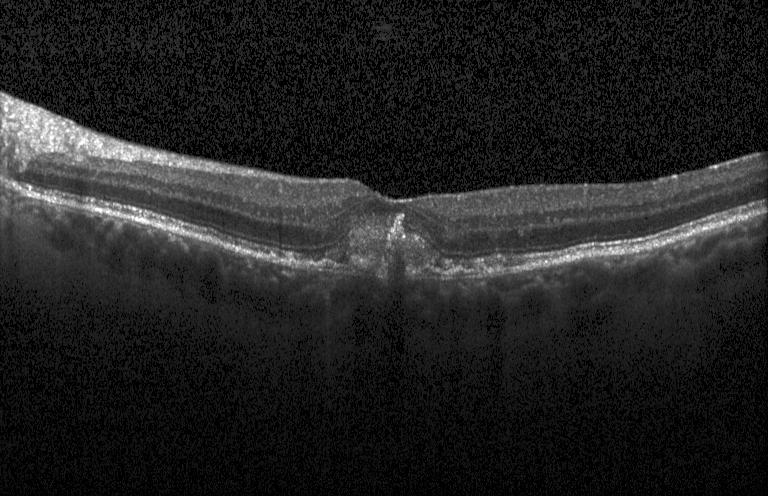 OCT scan showing a choroidal neovascular membrane.